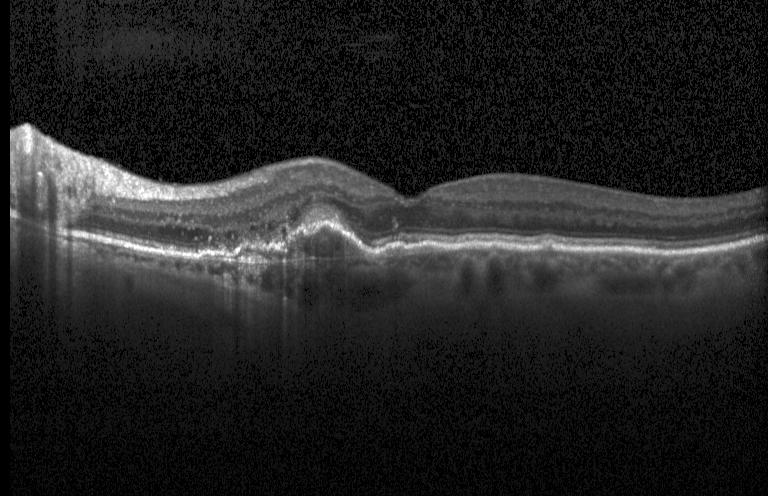
Optical coherence tomography scan · spectral-domain optical coherence tomography
A choroidal neovascular membrane.